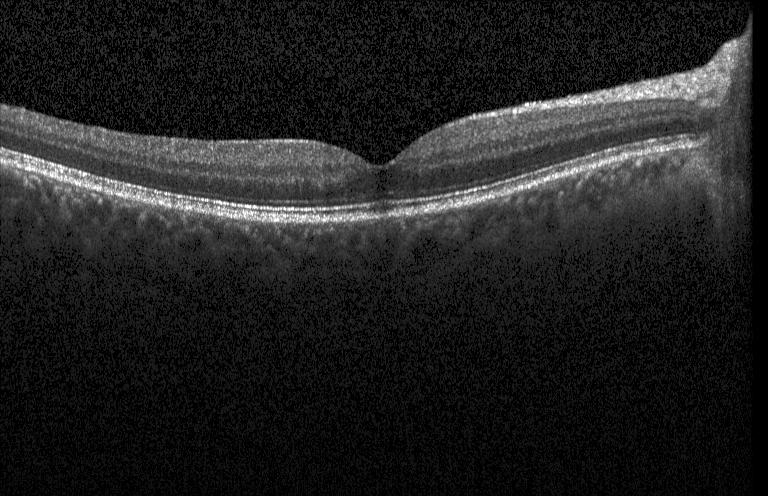 Macular OCT: no choroidal neovascularization, diabetic macular edema, or drusen.